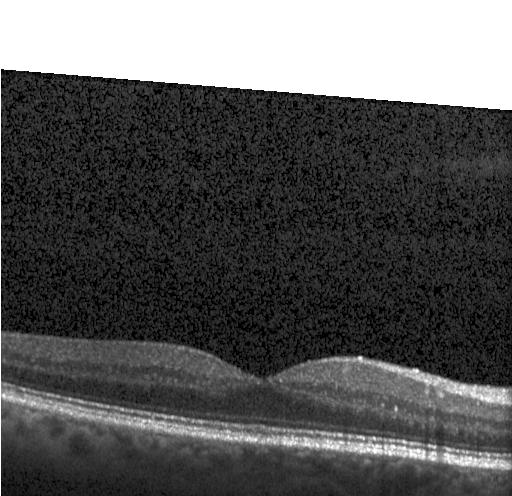 OCT line scan — Diagnosis: no choroidal neovascularization, diabetic macular edema, or drusen.